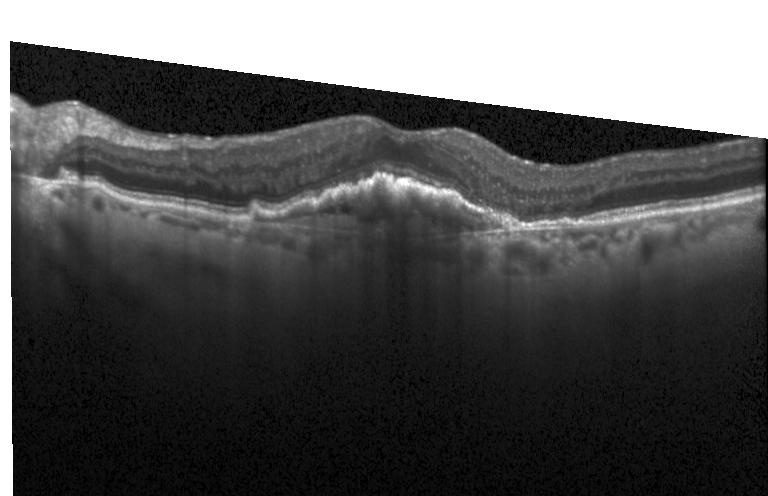 Spectral-domain OCT. Horizontal scan through the fovea. Optical coherence tomography scan. Impression: CNV.